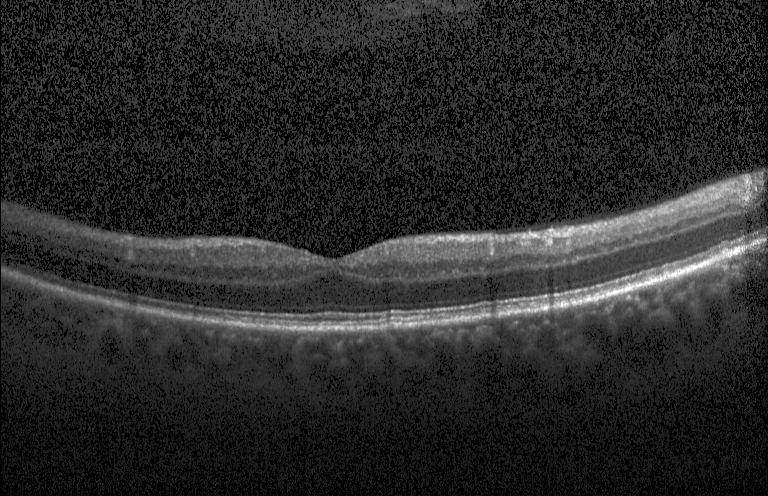

OCT finding: no choroidal neovascularization, diabetic macular edema, or drusen.